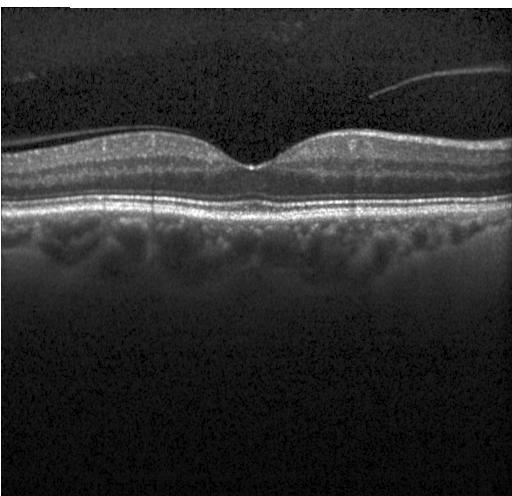

Retinal OCT cross-section. Finding: no evidence of choroidal neovascularization, diabetic macular edema, or drusen.